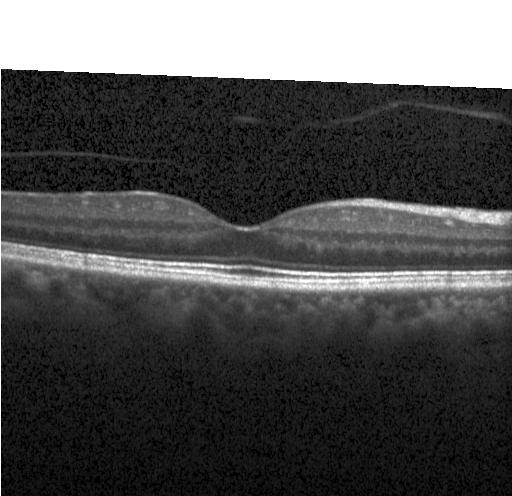
OCT scan showing neither choroidal neovascularization, diabetic macular edema, nor drusen.